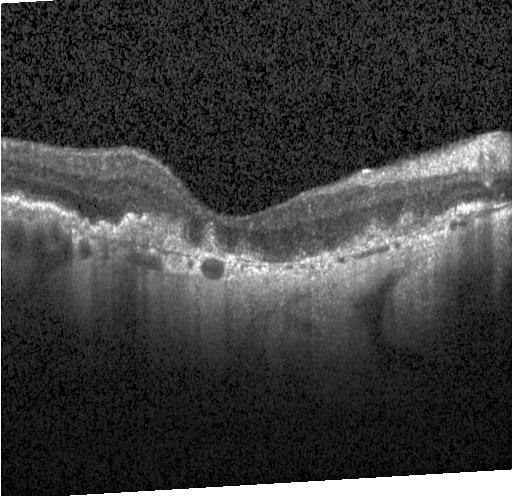

Heidelberg Spectralis OCT system. OCT B-scan. Diagnosis: a choroidal neovascular membrane.